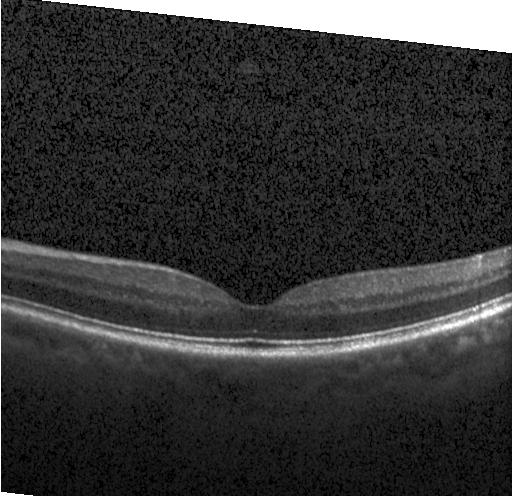 Acquired on a Heidelberg Spectralis; OCT line scan; spectral-domain OCT. OCT finding: neither choroidal neovascularization, diabetic macular edema, nor drusen.